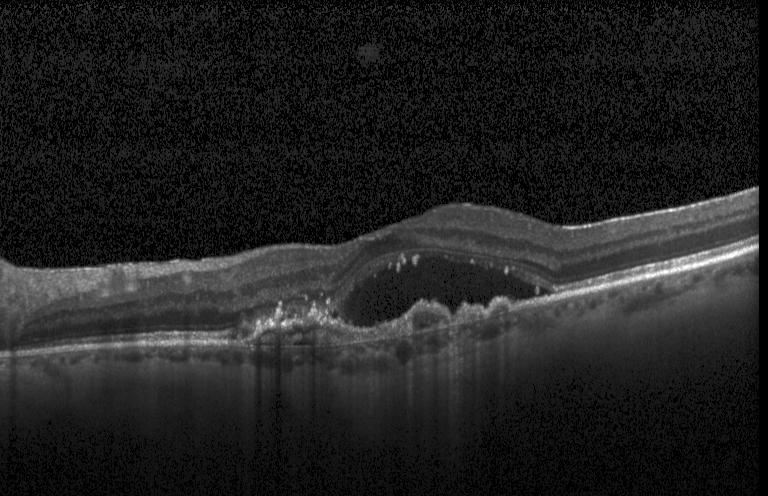

Acquired on a Heidelberg Spectralis. Spectral-domain OCT. Through the macula. Retinal OCT cross-section — Diagnosis: CNV.